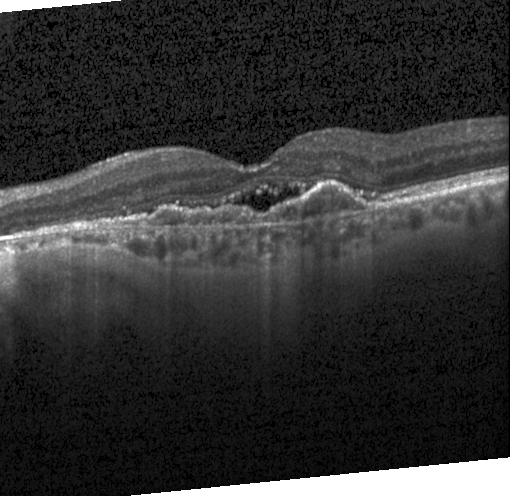

Diagnosis: CNV.